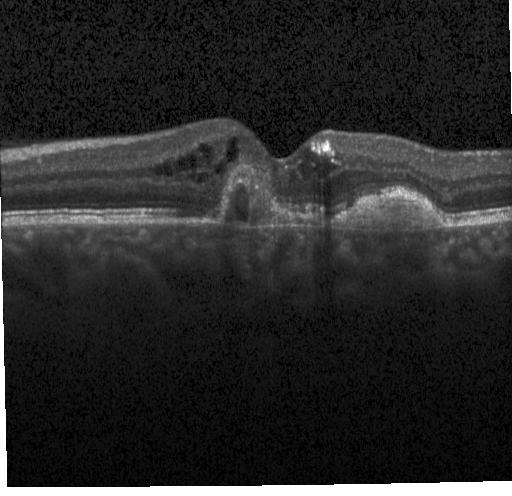
OCT finding: choroidal neovascularization (CNV).